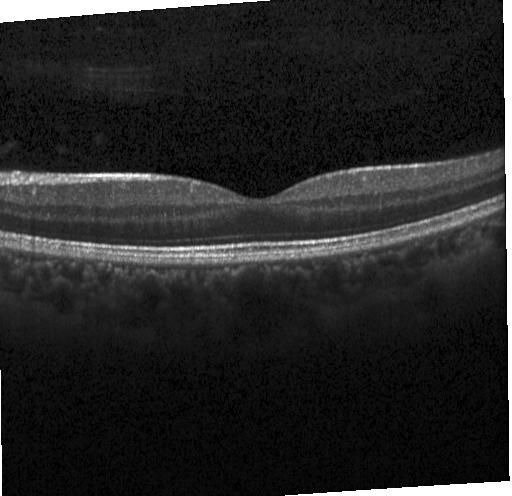 Retinal OCT B-scan.
Assessment: no evidence of CNV, DME, or drusen.